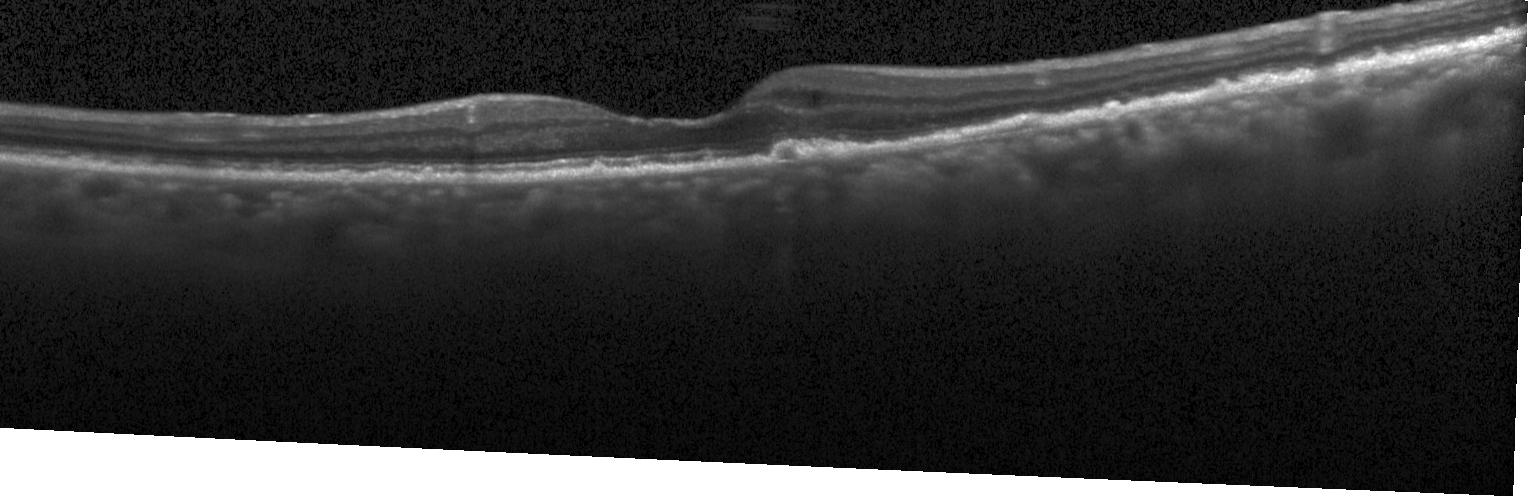
Diagnosis: a choroidal neovascular membrane.